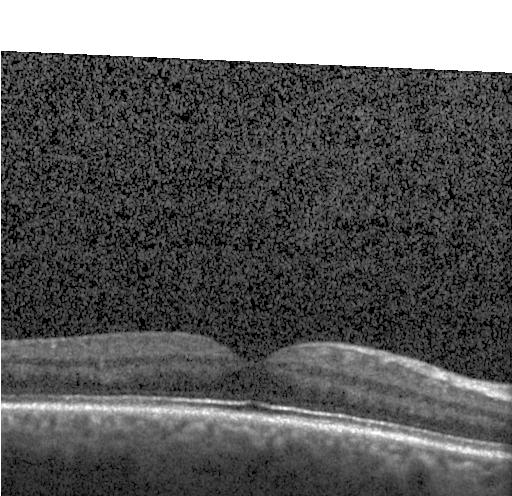

OCT line scan; spectral-domain optical coherence tomography — Diagnosis: no choroidal neovascularization, diabetic macular edema, or drusen.